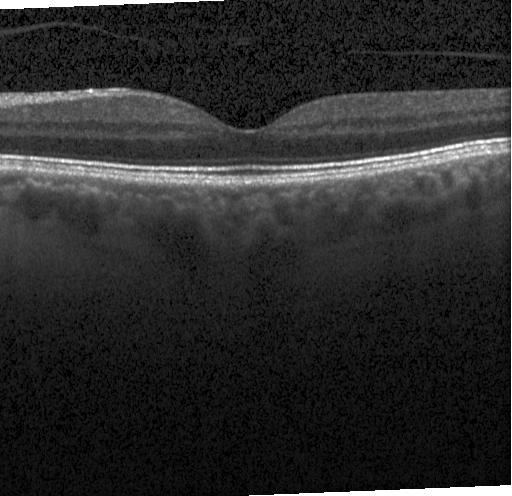

Finding: neither choroidal neovascularization, diabetic macular edema, nor drusen.